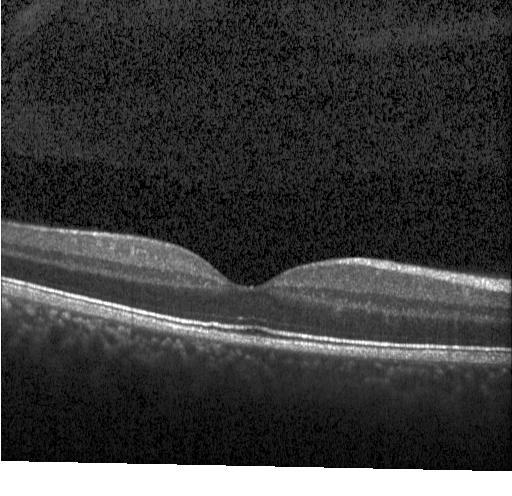
Spectral-domain OCT B-scan: neither choroidal neovascularization, diabetic macular edema, nor drusen.